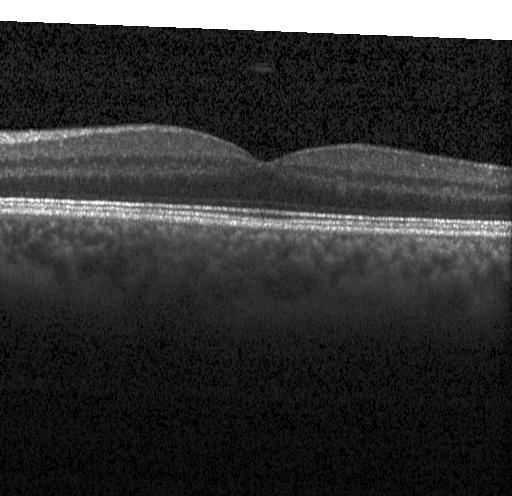
Acquired on a Heidelberg Spectralis; optical coherence tomography B-scan; SD-OCT — OCT finding: no choroidal neovascularization, no diabetic macular edema, and no drusen.